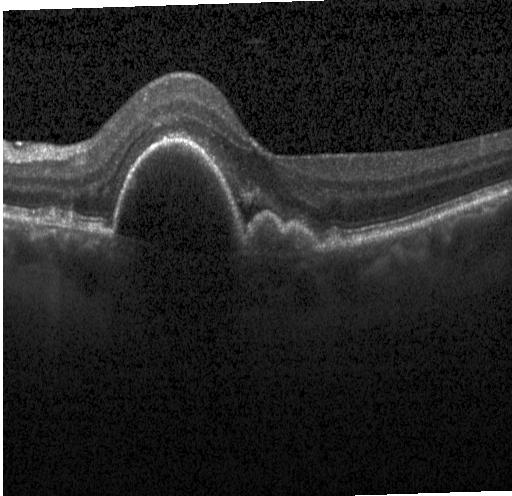

Retinal OCT cross-section. Impression: CNV.